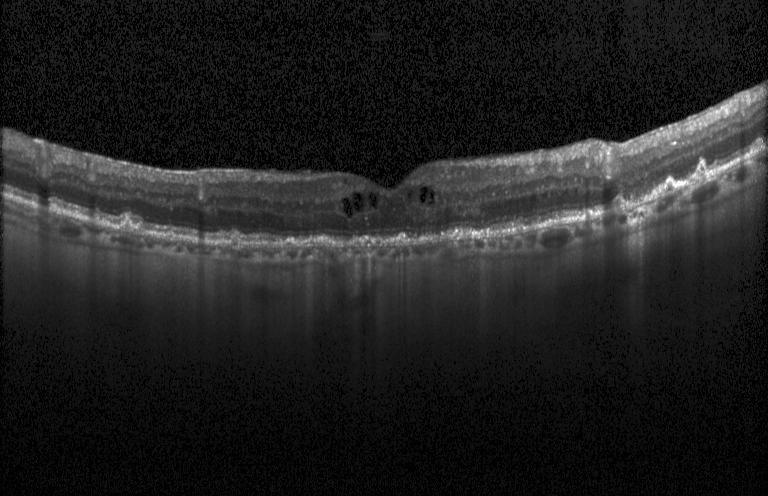 OCT line scan. SD-OCT — Impression: a choroidal neovascular membrane.